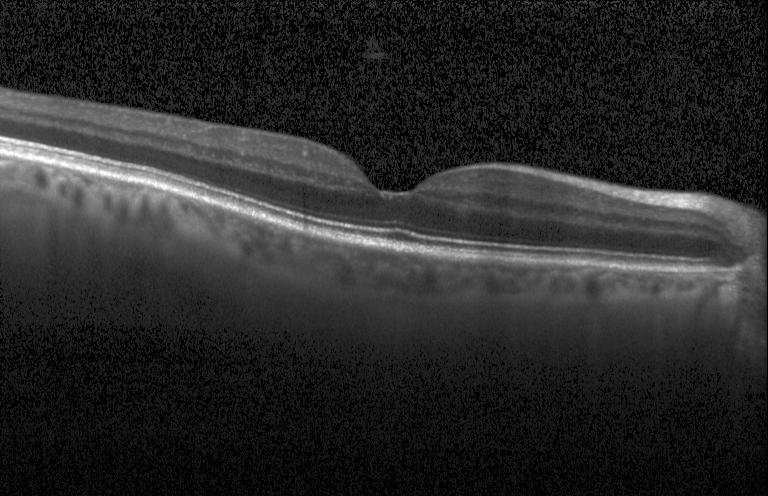
Heidelberg Spectralis OCT system. Centered on the fovea. Optical coherence tomography scan. Spectral-domain OCT — This B-scan demonstrates no evidence of choroidal neovascularization, diabetic macular edema, or drusen.